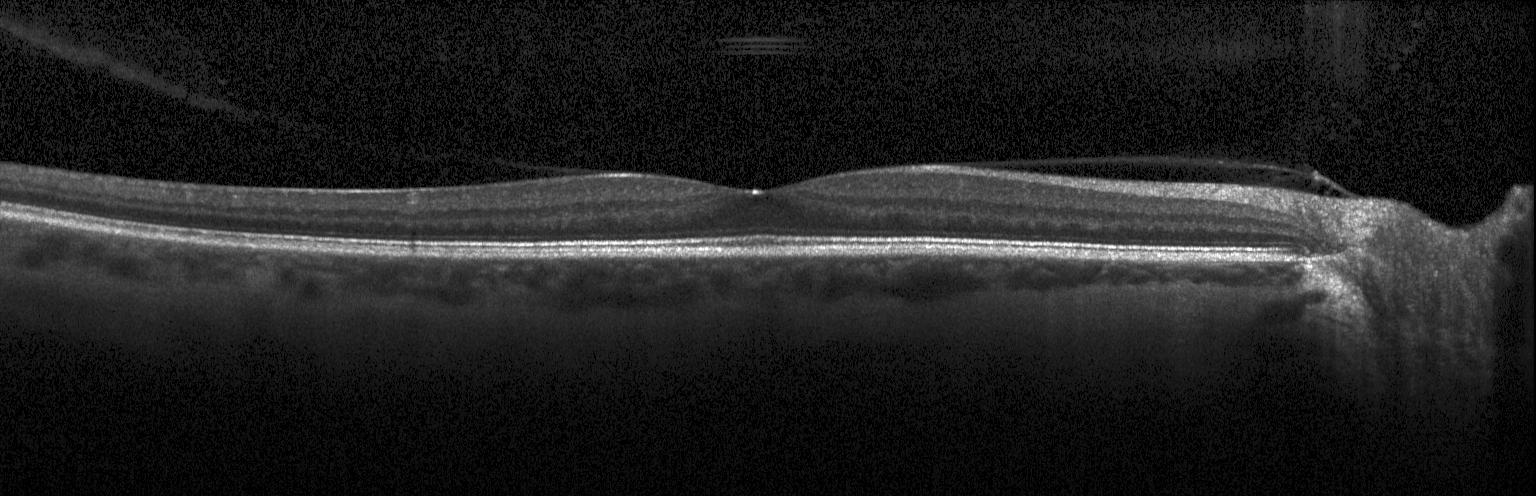
The scan shows no evidence of choroidal neovascularization, diabetic macular edema, or drusen.